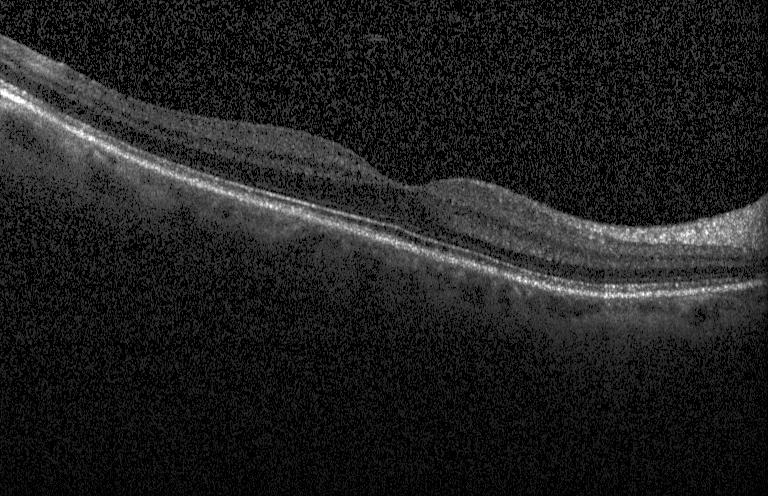
Macular scan; optical coherence tomography scan; acquired on a Heidelberg Spectralis; SD-OCT. Diagnosis: no choroidal neovascularization, no diabetic macular edema, and no drusen.